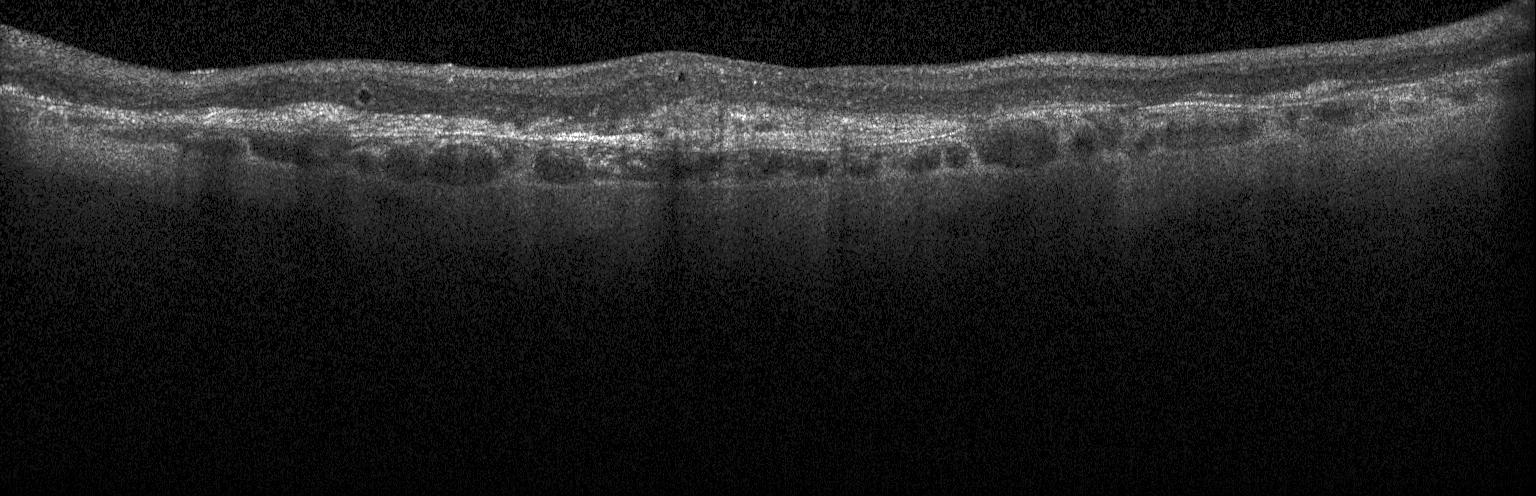

Optical coherence tomography B-scan
Impression: CNV.